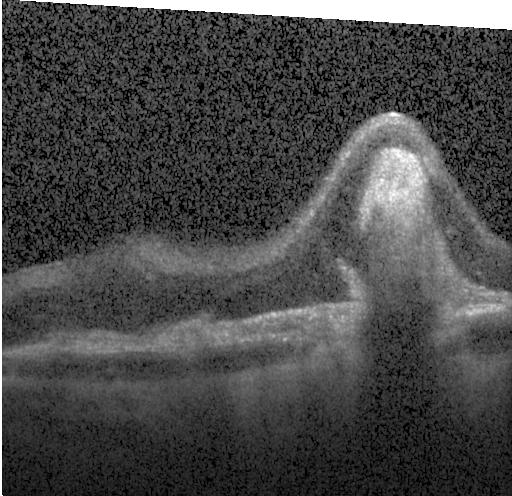 Diagnosis: a choroidal neovascular membrane.